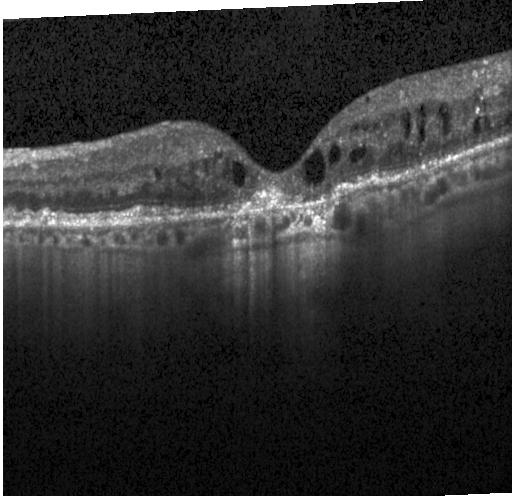
Optical coherence tomography B-scan
Macular OCT: a choroidal neovascular membrane.